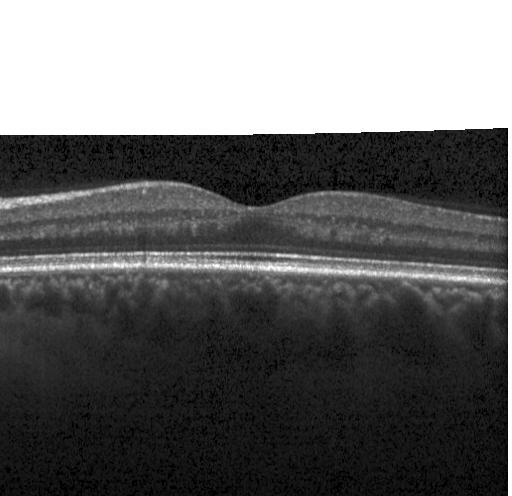

Retinal OCT cross-section. Impression: no choroidal neovascularization, no diabetic macular edema, and no drusen.